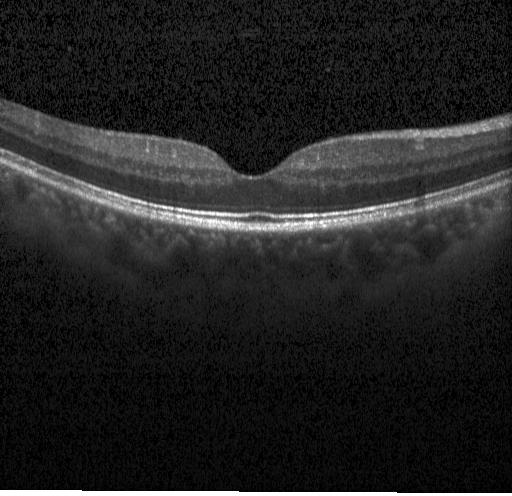
OCT line scan, horizontal scan through the fovea. This B-scan demonstrates no choroidal neovascularization, no diabetic macular edema, and no drusen.